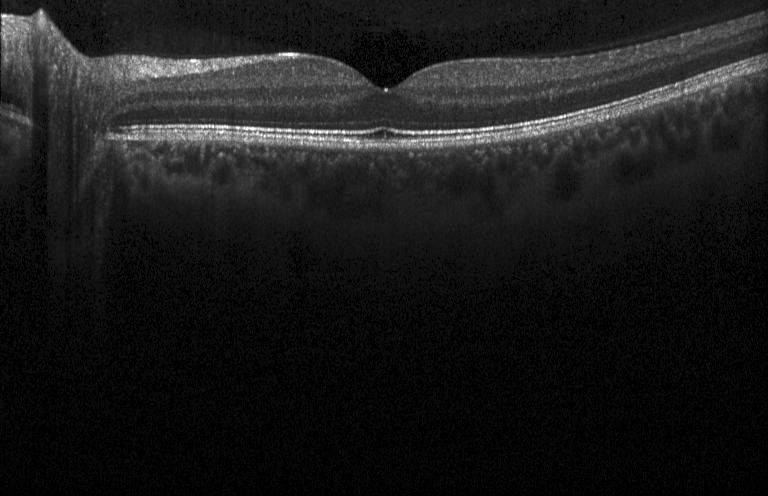
Finding: no CNV, no DME, and no drusen.